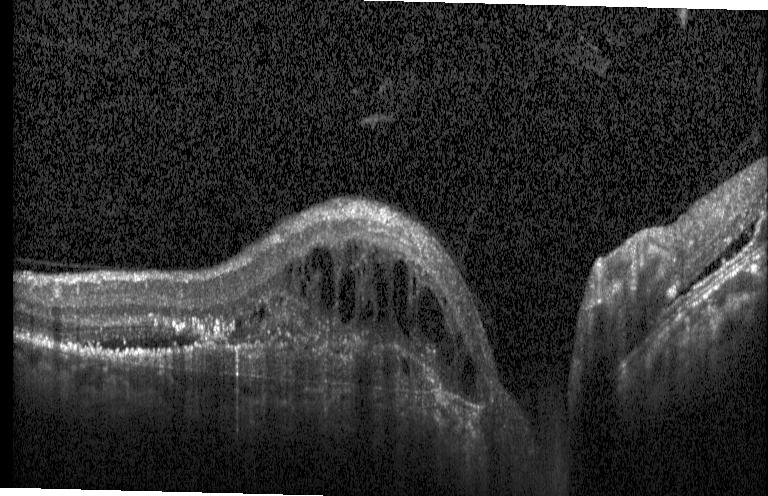 OCT scan showing a choroidal neovascular membrane.